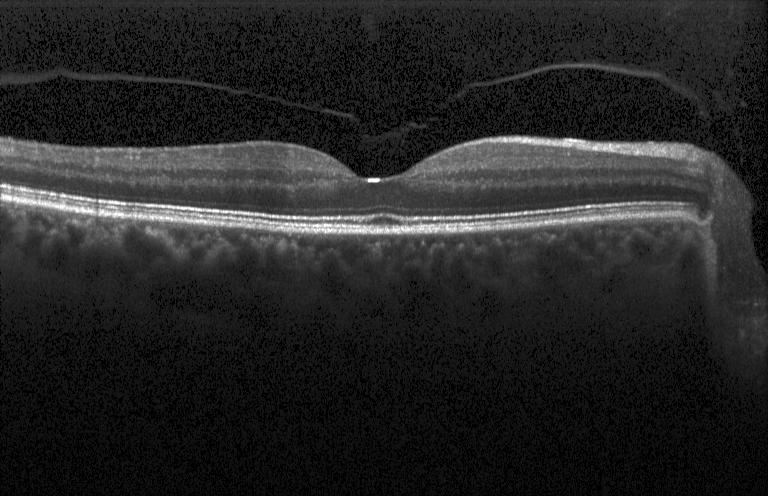 Finding: neither CNV, DME, nor drusen.